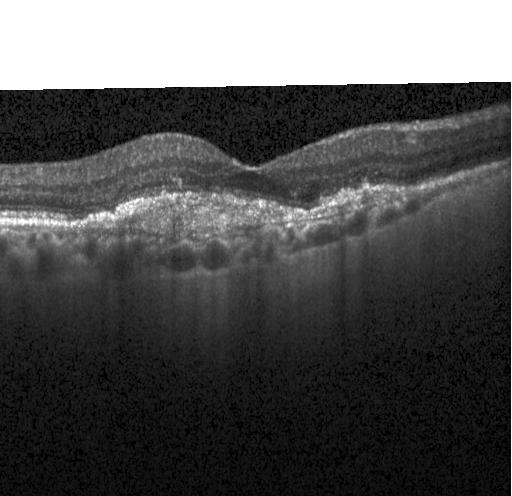 Retinal OCT B-scan — The scan shows choroidal neovascularization (CNV).